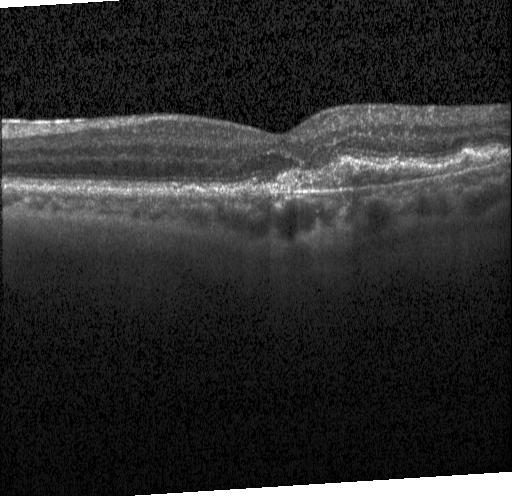
Retinal OCT B-scan; Heidelberg Spectralis; centered on the fovea. Impression: CNV.